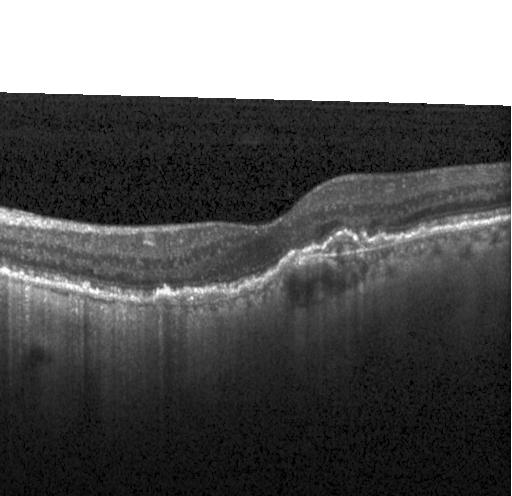

Through the macula · OCT line scan · spectral-domain OCT · acquired on a Heidelberg Spectralis
OCT finding: a choroidal neovascular membrane.